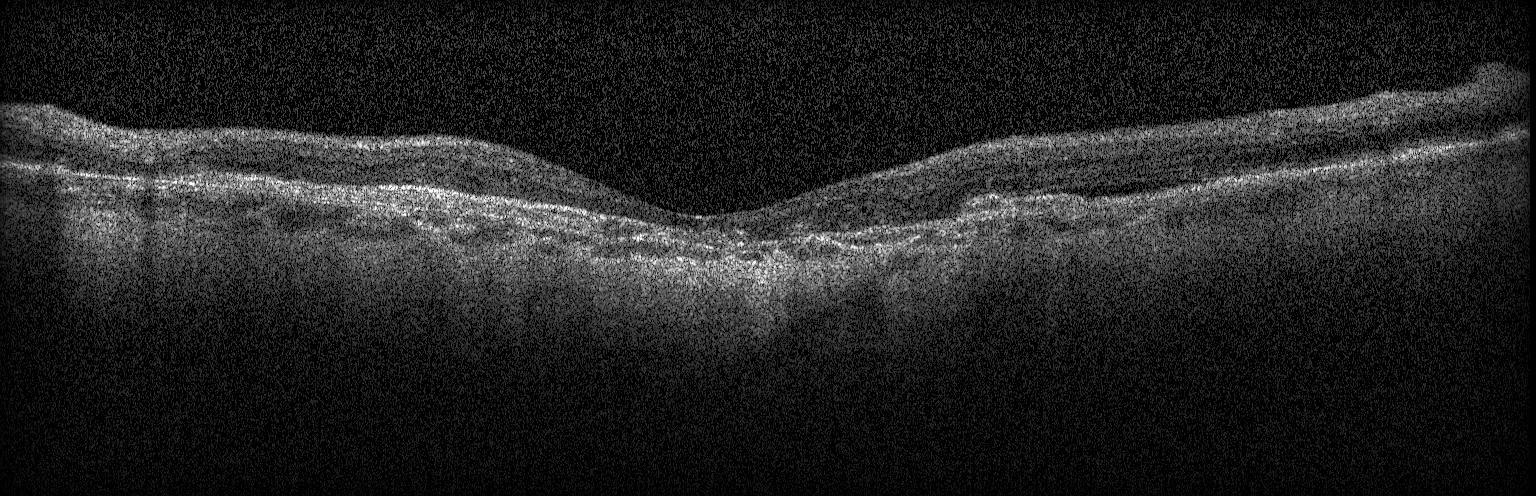
Heidelberg Spectralis; retinal OCT B-scan; spectral-domain OCT; through the macula.
Diagnosis: a choroidal neovascular membrane.